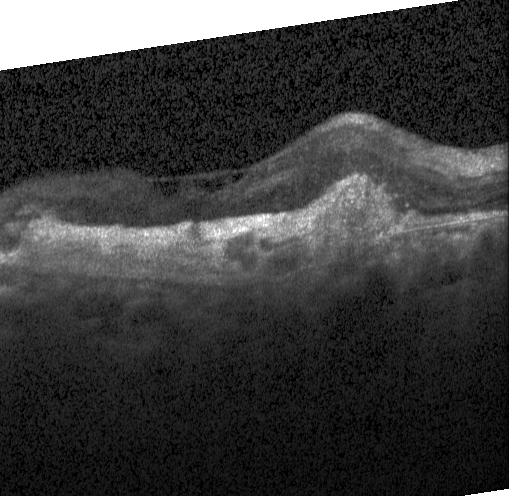 Through the macula. Spectral-domain OCT. Optical coherence tomography scan. Heidelberg Spectralis OCT system. Macular OCT: CNV.